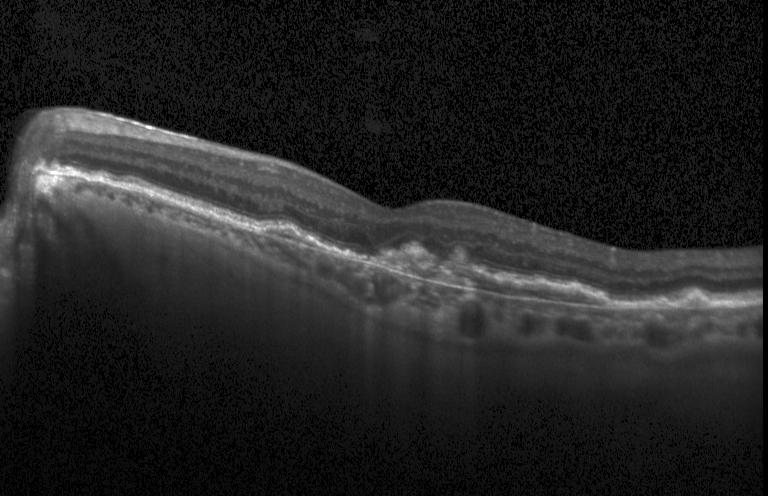

Spectral-domain optical coherence tomography, horizontal scan through the fovea, optical coherence tomography scan, acquired on a Heidelberg Spectralis — Dx: choroidal neovascularization.